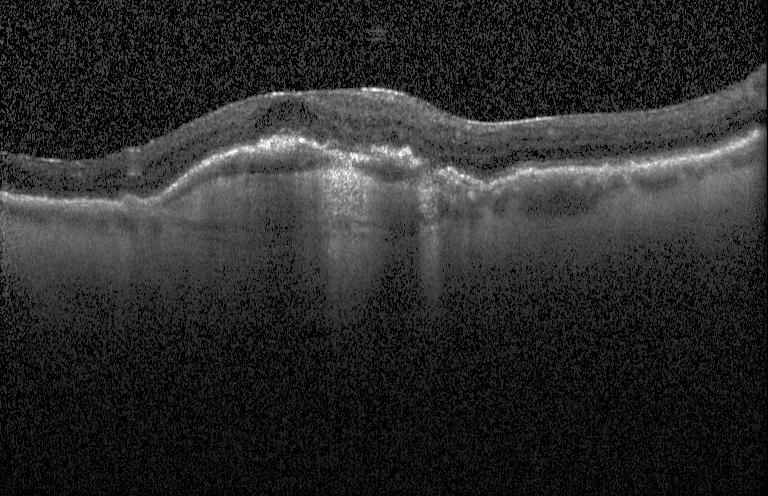

Optical coherence tomography scan. This B-scan demonstrates choroidal neovascularization.